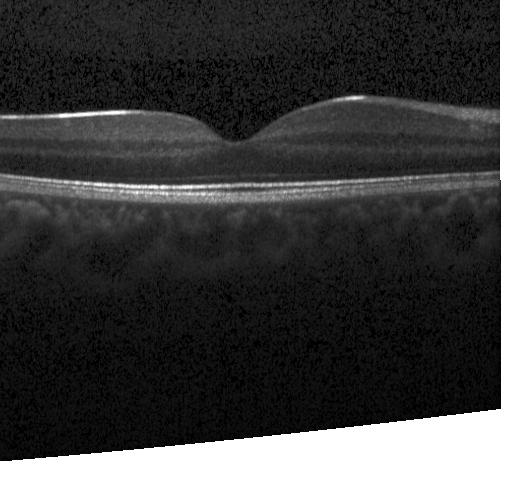
Spectral-domain OCT. OCT line scan — Dx: no CNV, DME, or drusen.